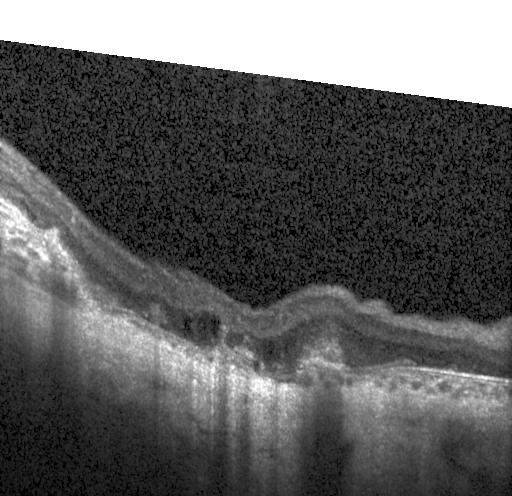

Horizontal scan through the fovea · retinal OCT cross-section · spectral-domain optical coherence tomography
Finding: CNV.